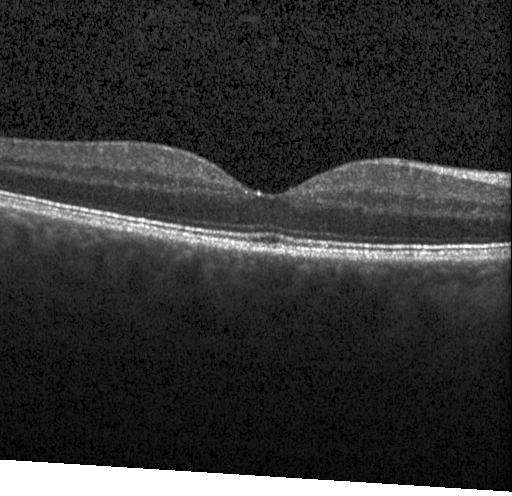 Impression: no choroidal neovascularization, diabetic macular edema, or drusen.